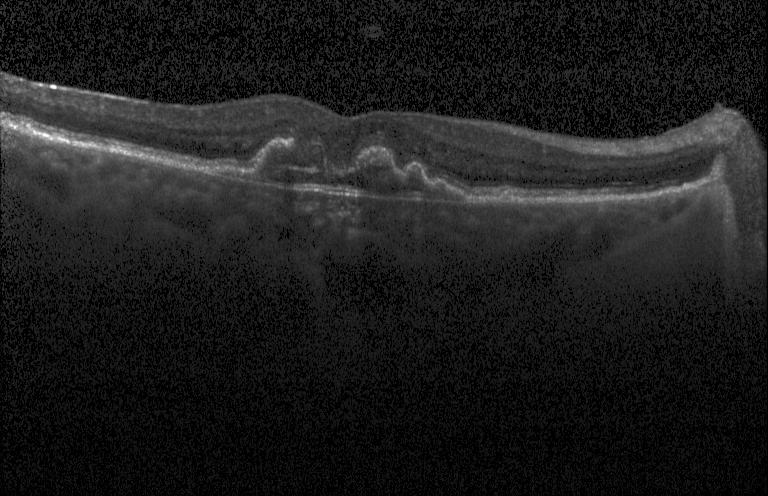 OCT B-scan. Assessment: CNV.